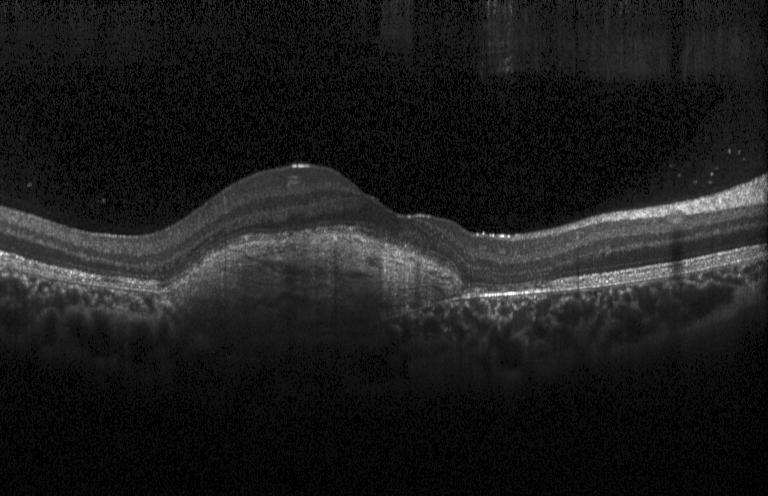 Diagnosis: a choroidal neovascular membrane.